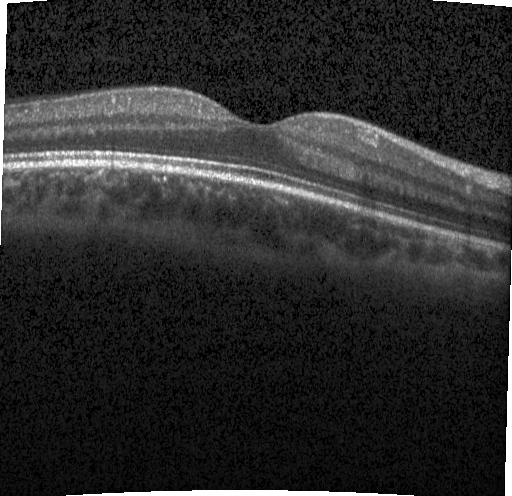

Diagnosis: neither choroidal neovascularization, diabetic macular edema, nor drusen.